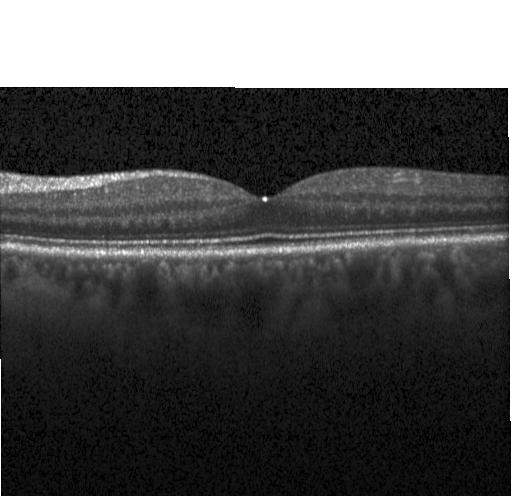

Spectral-domain OCT B-scan: no evidence of CNV, DME, or drusen.